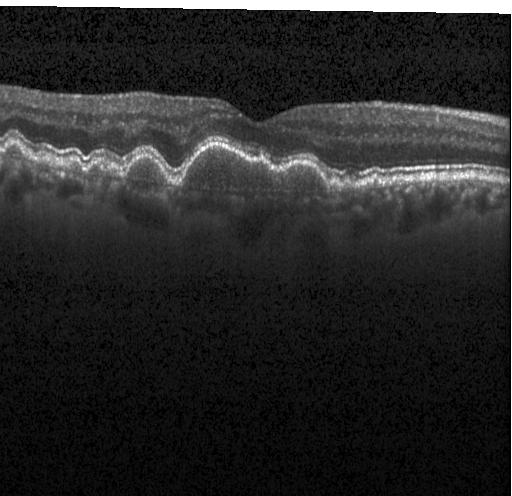

OCT B-scan
The scan shows multiple drusen.